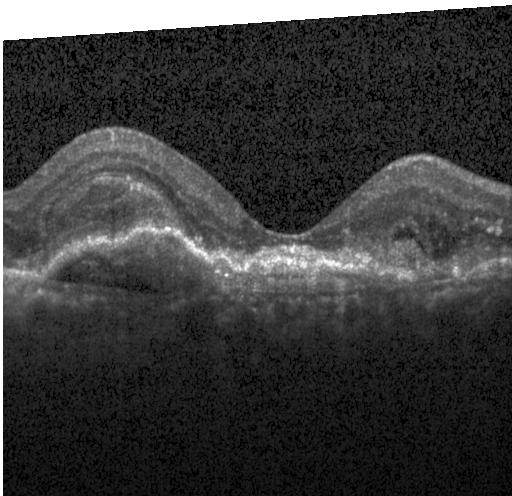 Optical coherence tomography scan; spectral-domain OCT; Heidelberg Spectralis; fovea-centered.
This B-scan demonstrates choroidal neovascularization.